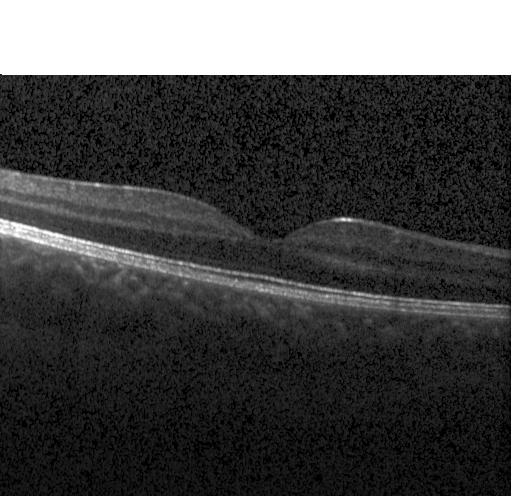
Optical coherence tomography scan; fovea-centered; SD-OCT; Heidelberg Spectralis. Impression: neither choroidal neovascularization, diabetic macular edema, nor drusen.